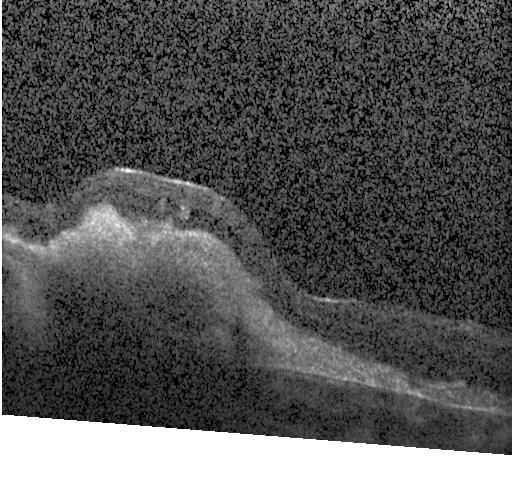
Macular OCT: choroidal neovascularization.